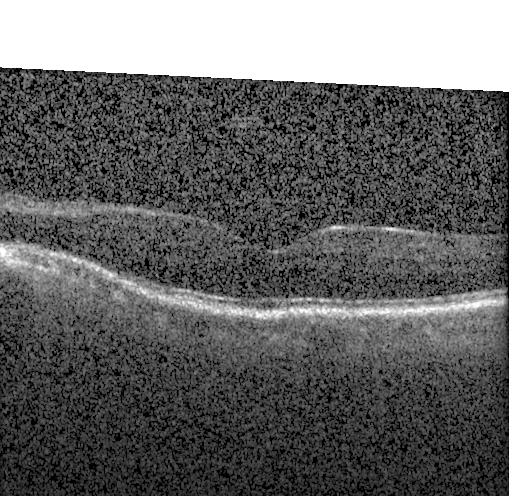
Impression: no choroidal neovascularization, no diabetic macular edema, and no drusen.